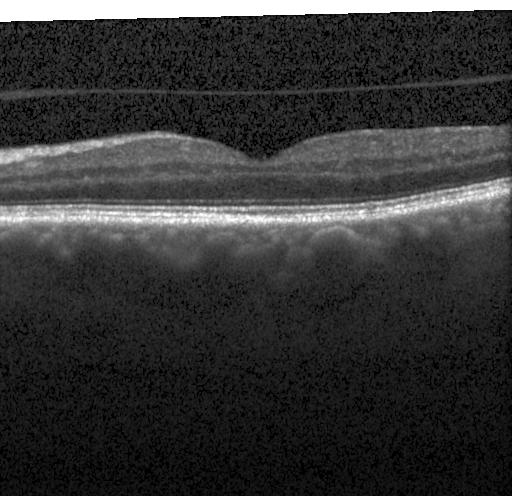

Impression: neither choroidal neovascularization, diabetic macular edema, nor drusen.